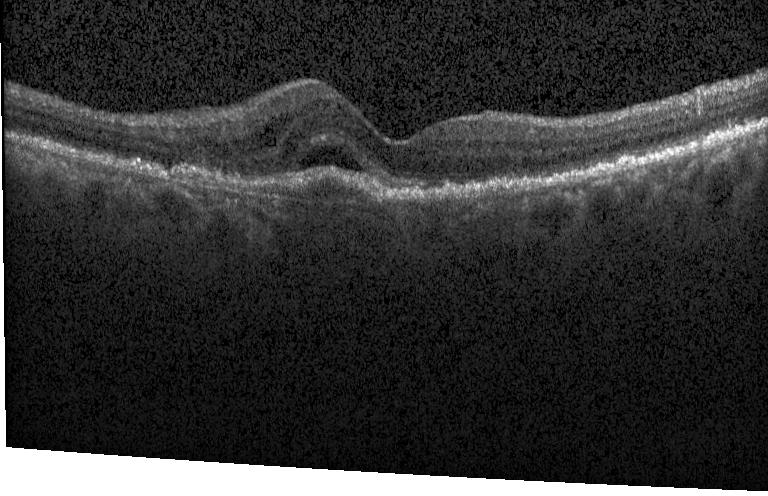 Spectral-domain optical coherence tomography, Heidelberg Spectralis OCT system, centered on the fovea, retinal OCT cross-section. A choroidal neovascular membrane.